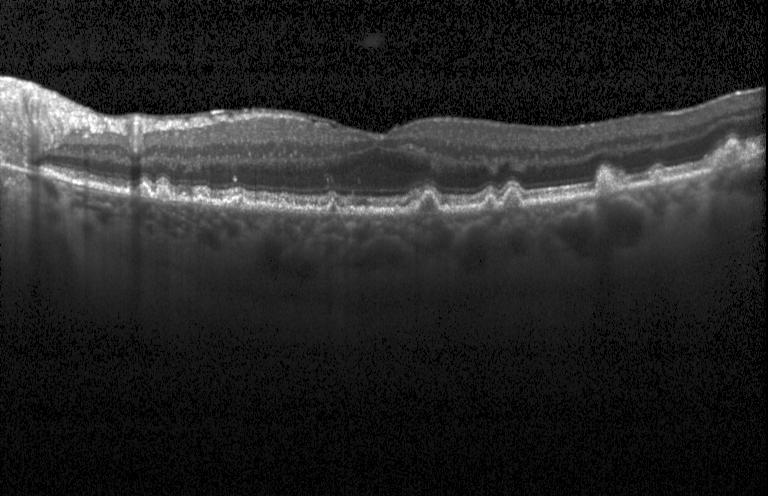 SD-OCT · instrument: Heidelberg Spectralis · centered on the fovea · optical coherence tomography scan.
Finding: sub-RPE drusenoid deposits.